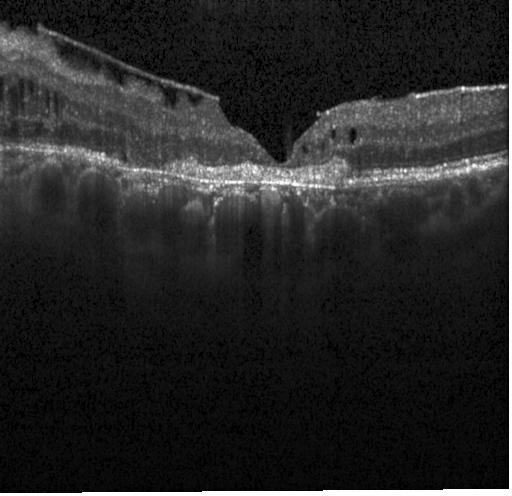

Through the macula. Retinal OCT B-scan. SD-OCT. Acquired on a Heidelberg Spectralis.
Finding: a choroidal neovascular membrane.